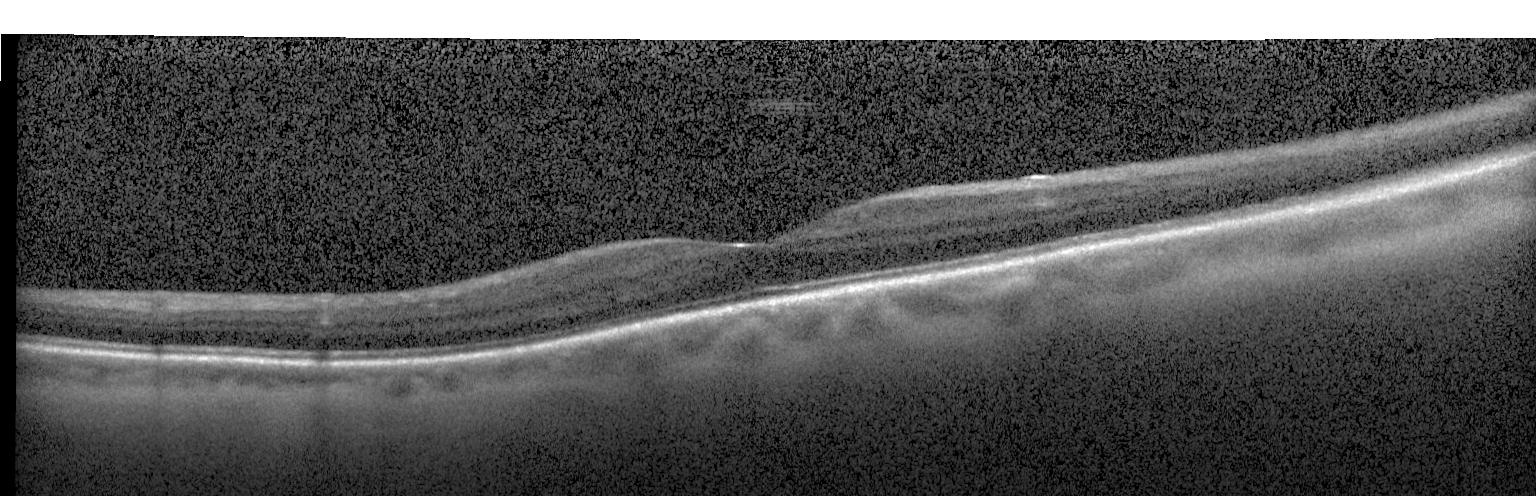

Optical coherence tomography B-scan. SD-OCT.
Diagnosis: no evidence of CNV, DME, or drusen.